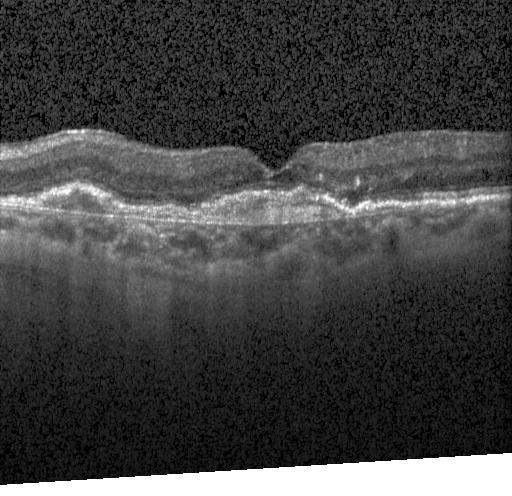
The scan shows CNV.